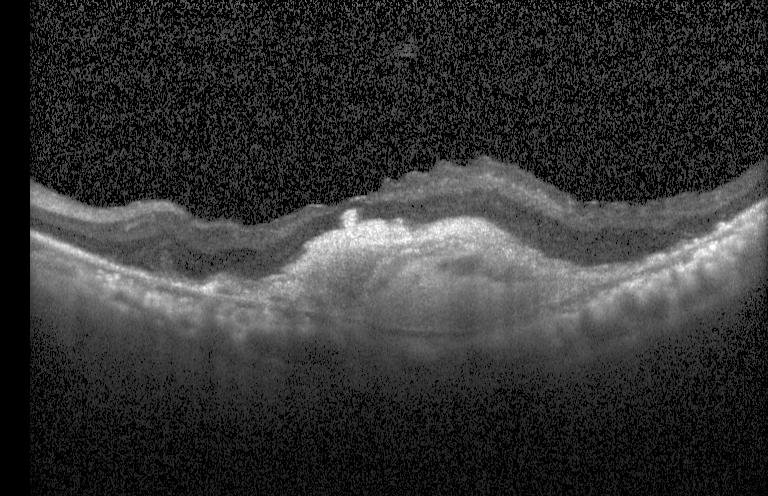

OCT B-scan · instrument: Heidelberg Spectralis. Choroidal neovascularization.